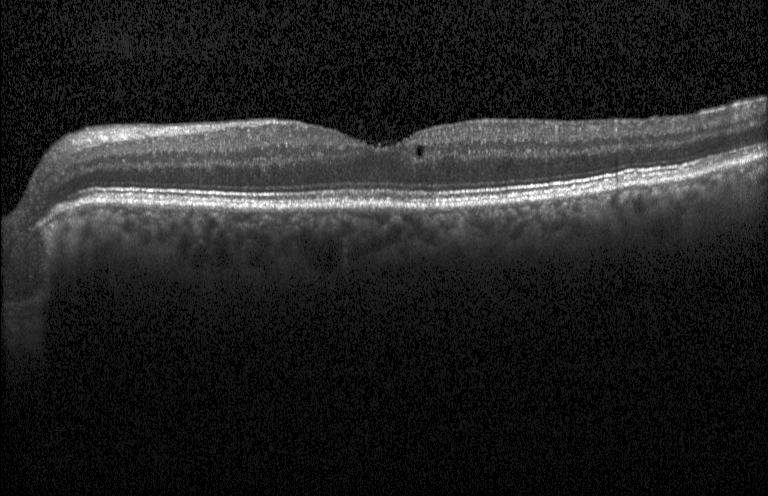 Macular scan. Optical coherence tomography scan — OCT finding: diabetic macular edema.